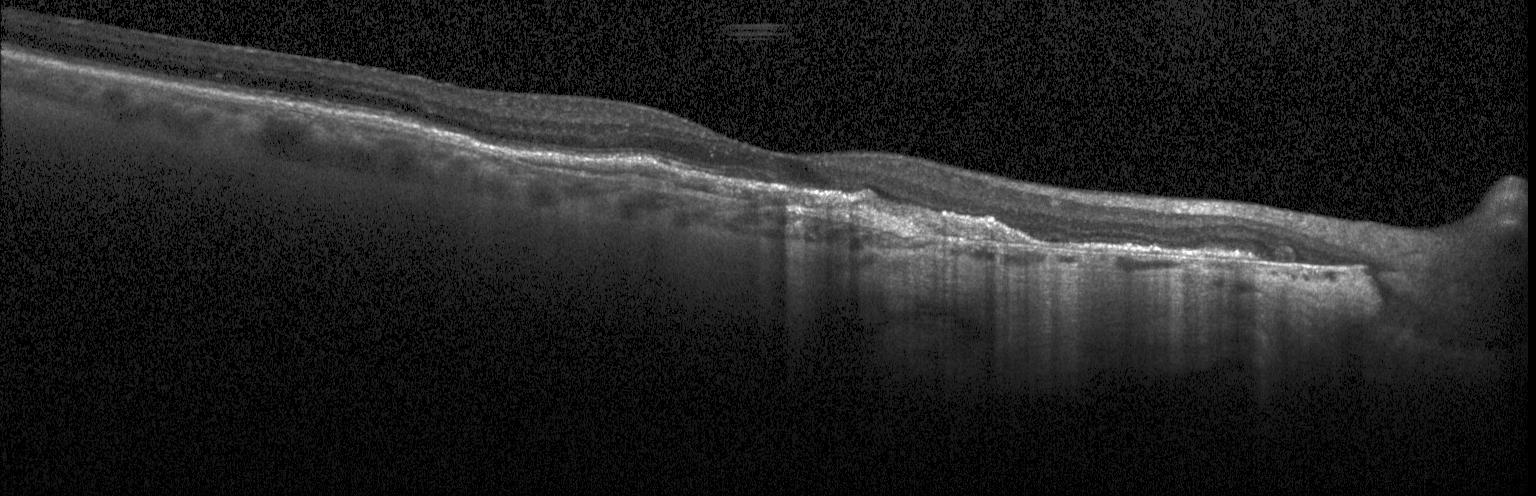 Impression: a choroidal neovascular membrane.